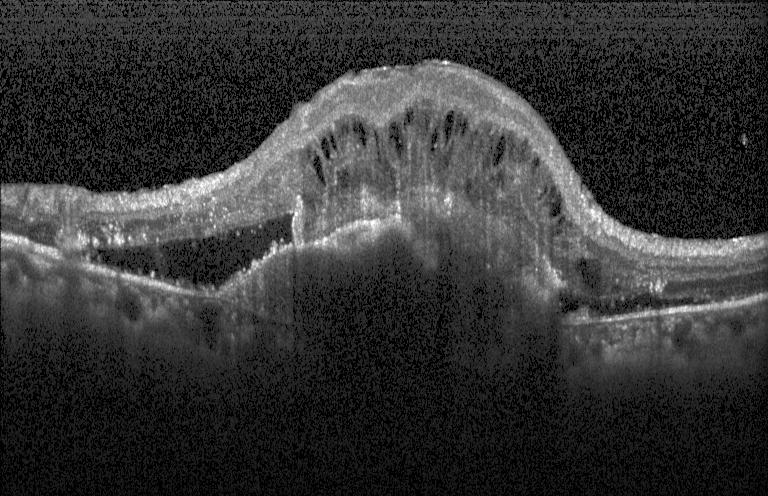 Heidelberg Spectralis; fovea-centered; optical coherence tomography B-scan; SD-OCT
Impression: choroidal neovascularization (CNV).